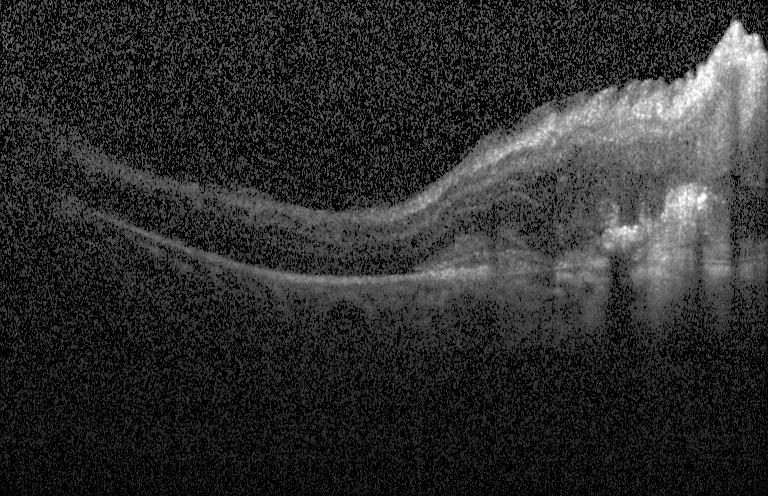 Retinal OCT cross-section; acquired on a Heidelberg Spectralis
Macular OCT: CNV.